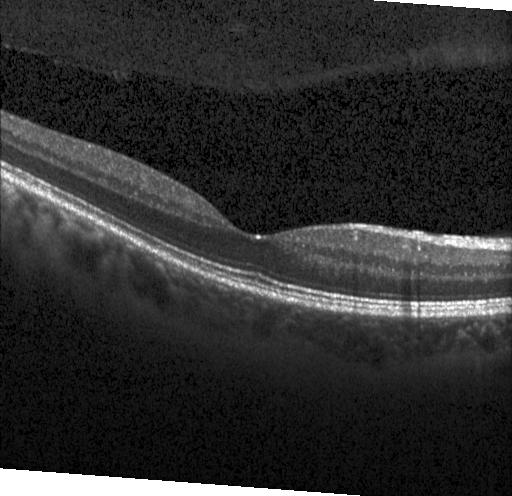
The scan shows neither CNV, DME, nor drusen.